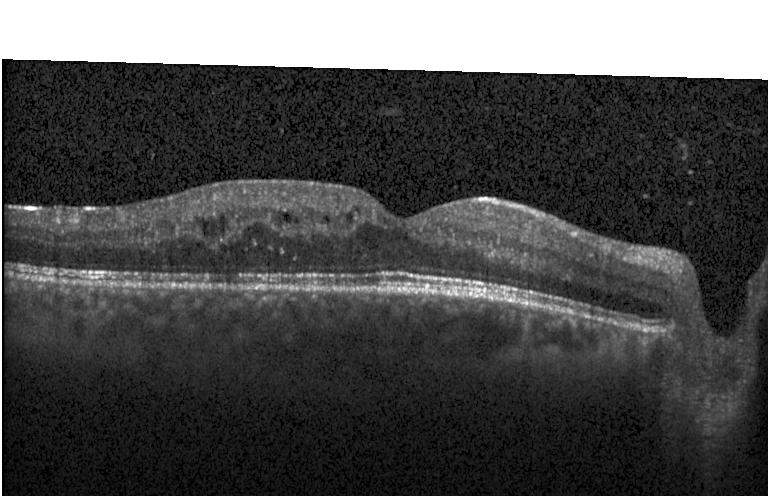

SD-OCT · horizontal scan through the fovea · instrument: Heidelberg Spectralis · OCT line scan.
Dx: diabetic macular edema (DME).